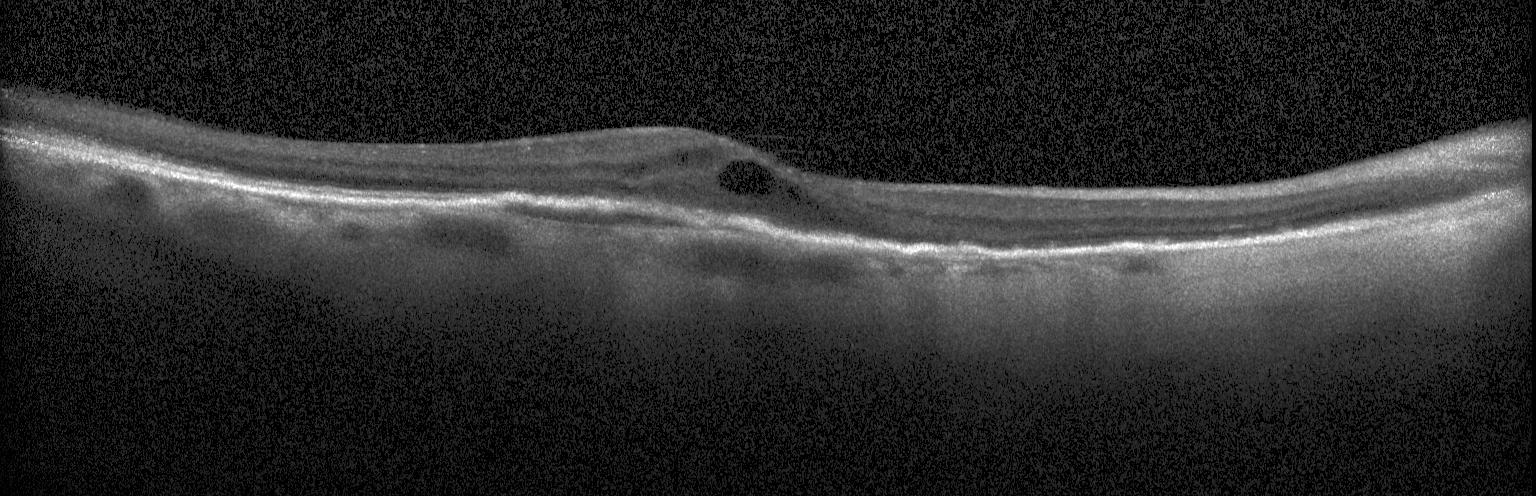
Macular OCT demonstrating choroidal neovascularization.